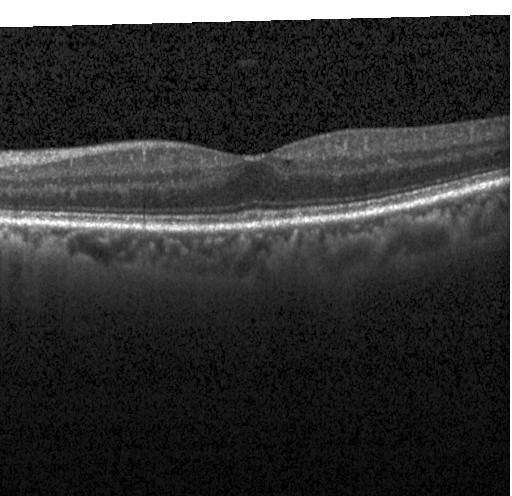

Assessment: neither choroidal neovascularization, diabetic macular edema, nor drusen.